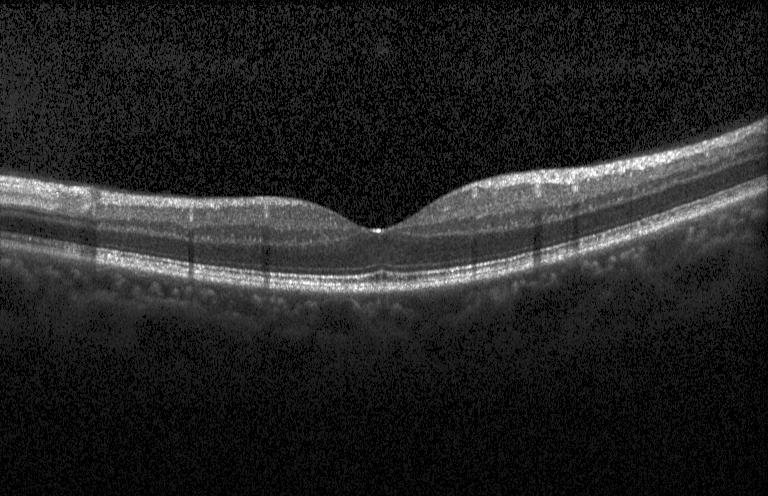
OCT B-scan showing no evidence of choroidal neovascularization, diabetic macular edema, or drusen.